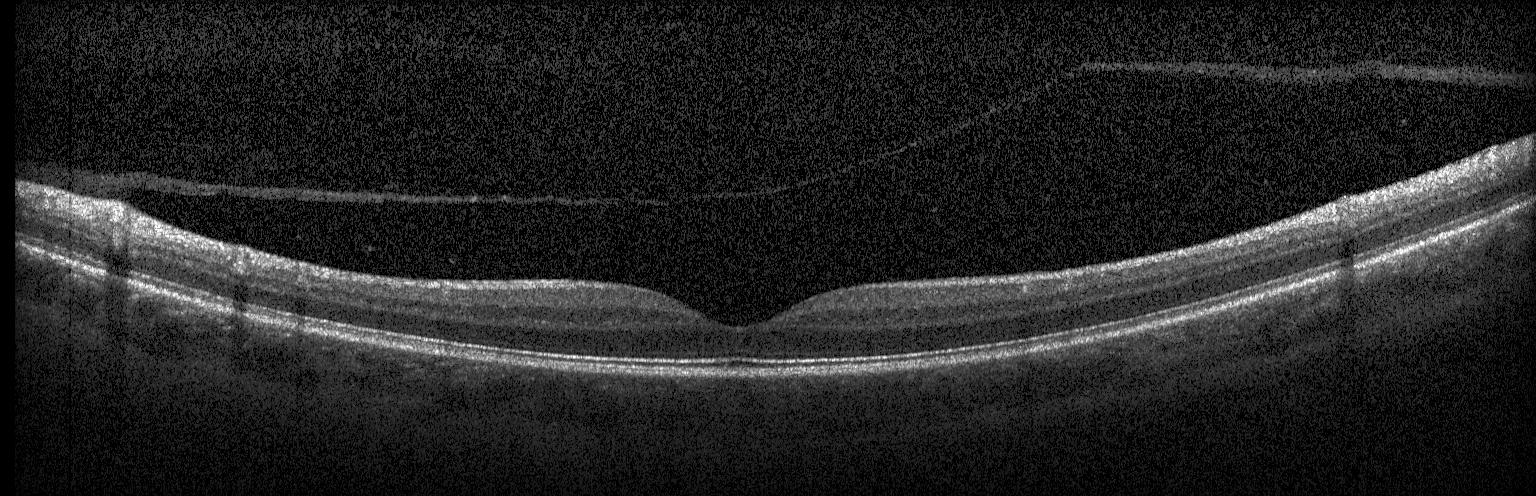

OCT B-scan. SD-OCT. Fovea-centered.
The scan shows no CNV, no DME, and no drusen.